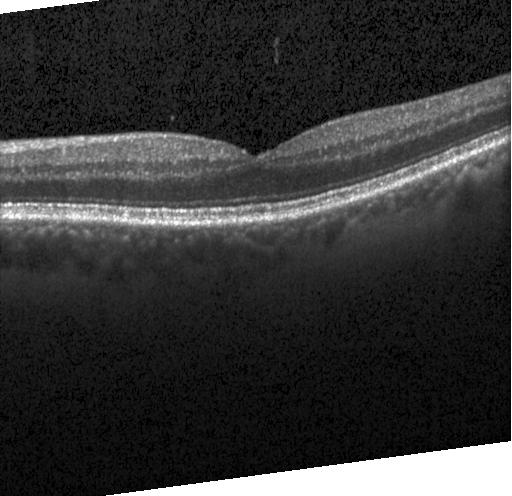

Impression: neither CNV, DME, nor drusen.